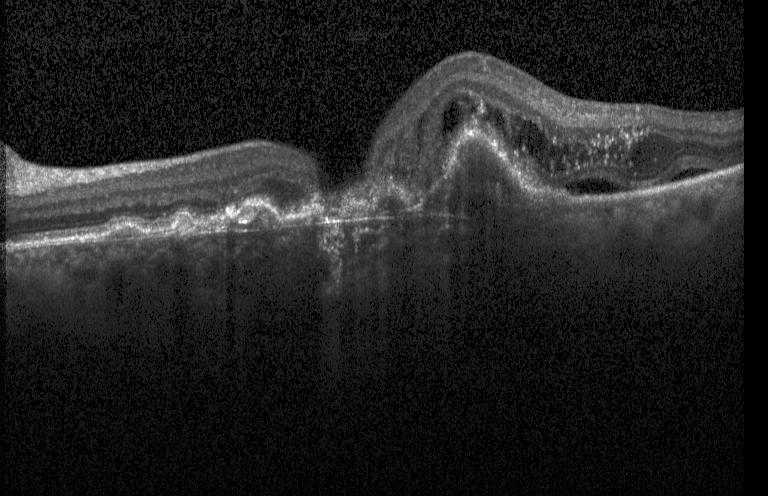 OCT B-scan. Impression: a choroidal neovascular membrane.